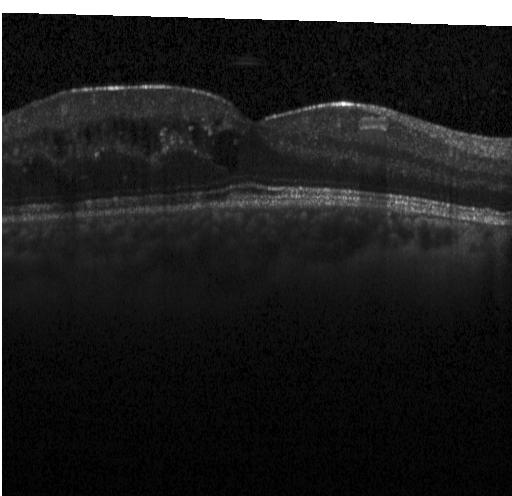

Diagnosis: diabetic macular edema.